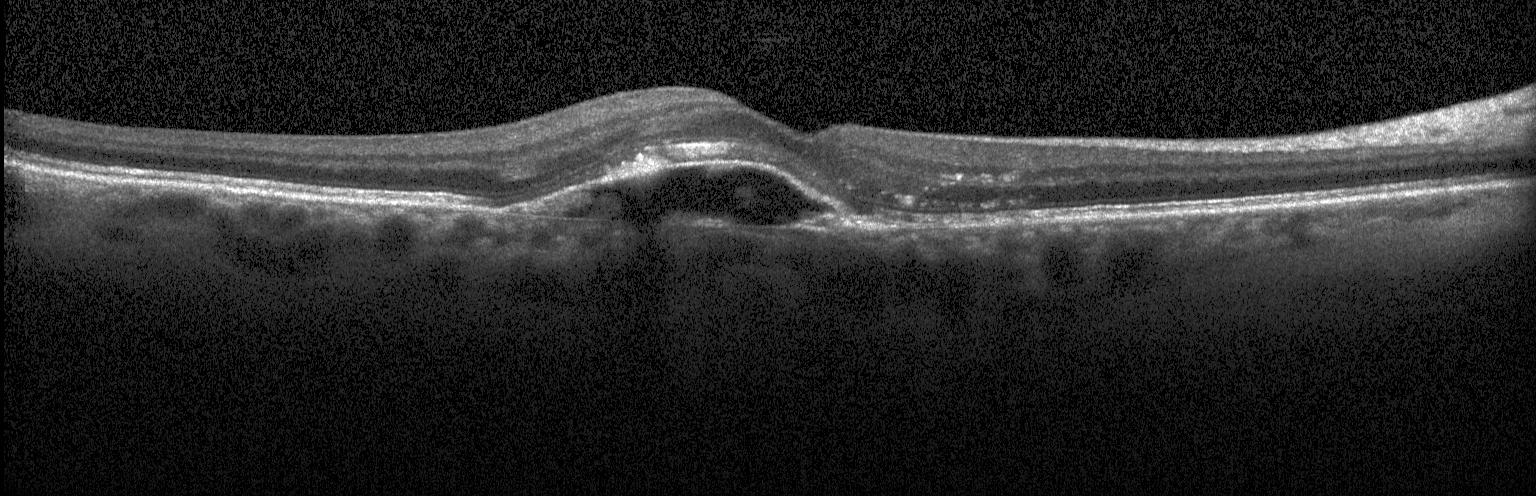

OCT scan showing choroidal neovascularization.